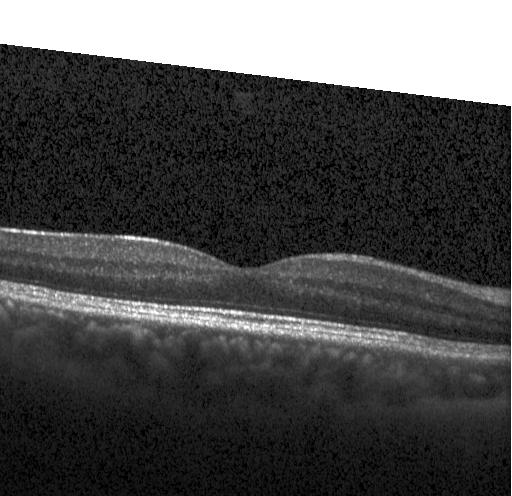
Impression: no evidence of choroidal neovascularization, diabetic macular edema, or drusen.